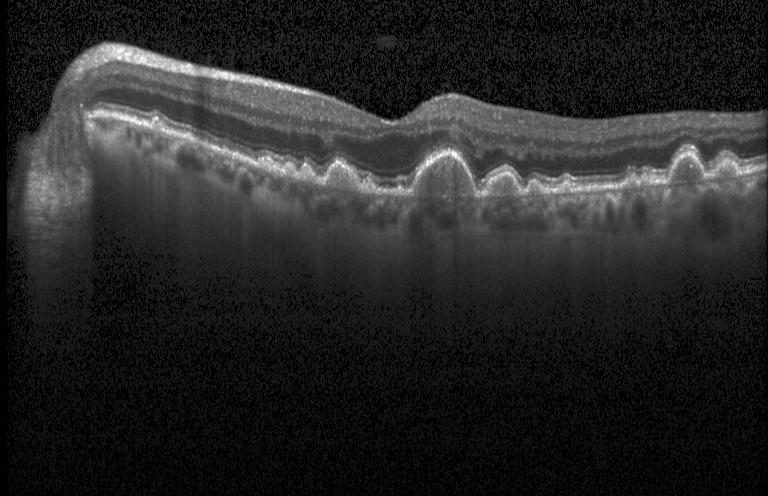 Sub-RPE drusenoid deposits.